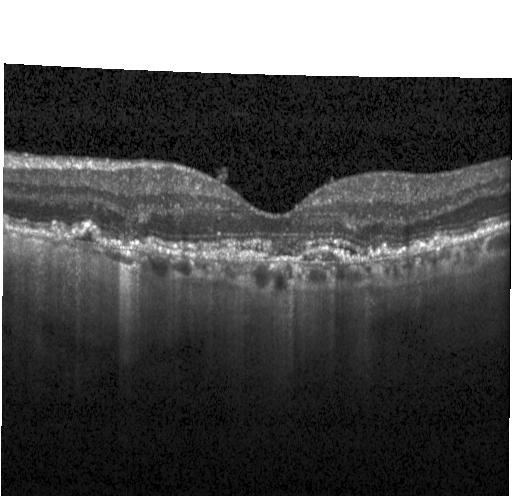

Impression: a choroidal neovascular membrane.